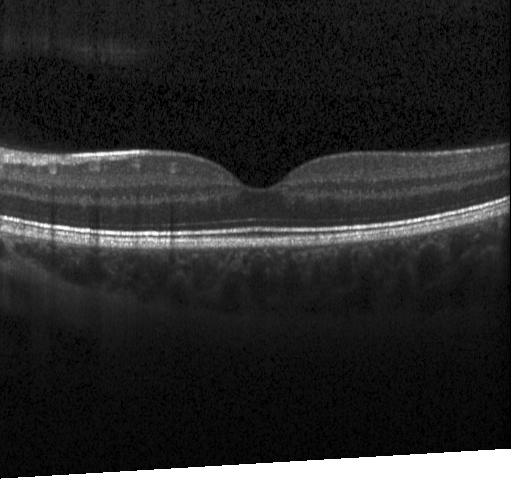 Spectral-domain OCT; retinal OCT cross-section; Heidelberg Spectralis — Neither choroidal neovascularization, diabetic macular edema, nor drusen.